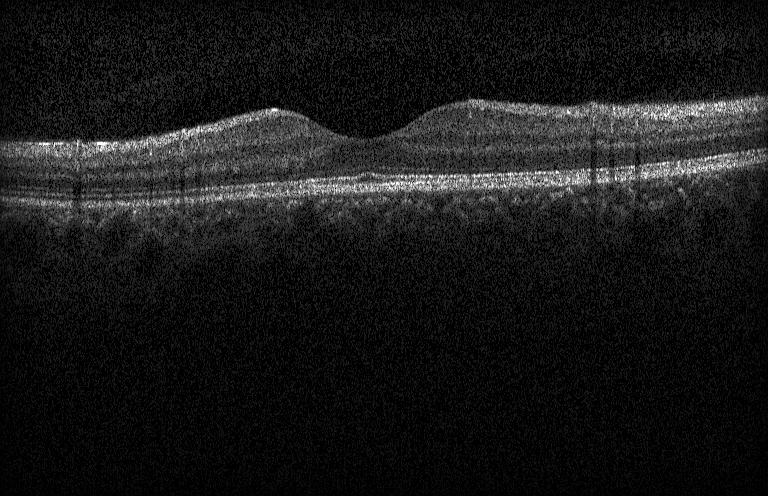 This B-scan demonstrates neither CNV, DME, nor drusen.